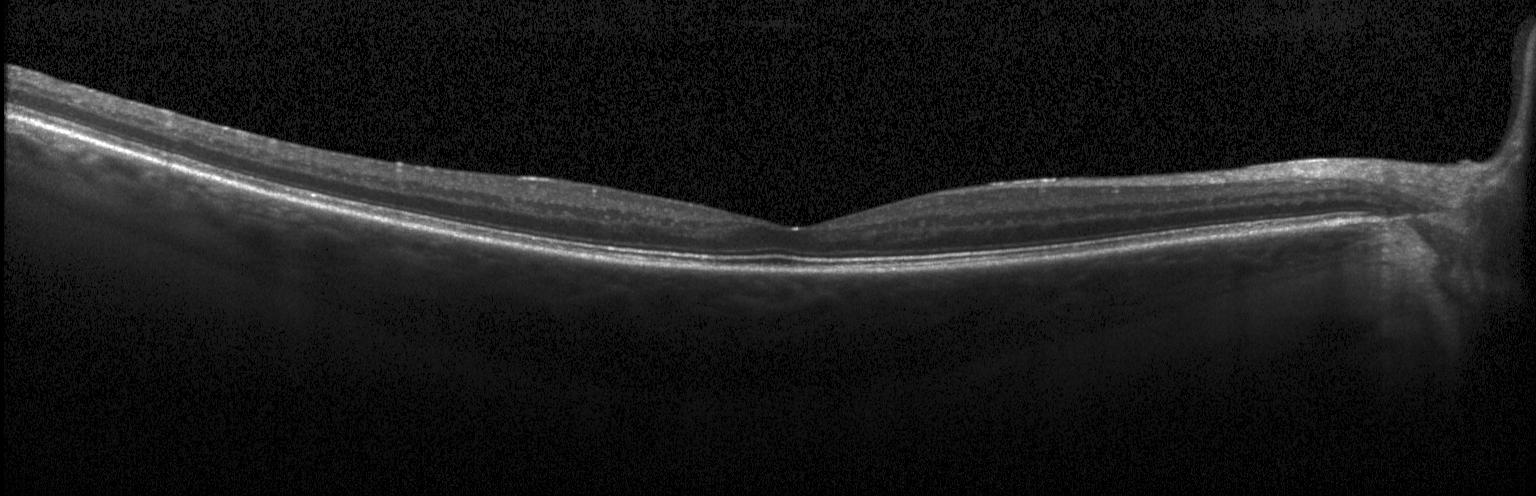 Optical coherence tomography B-scan. OCT finding: no choroidal neovascularization, diabetic macular edema, or drusen.